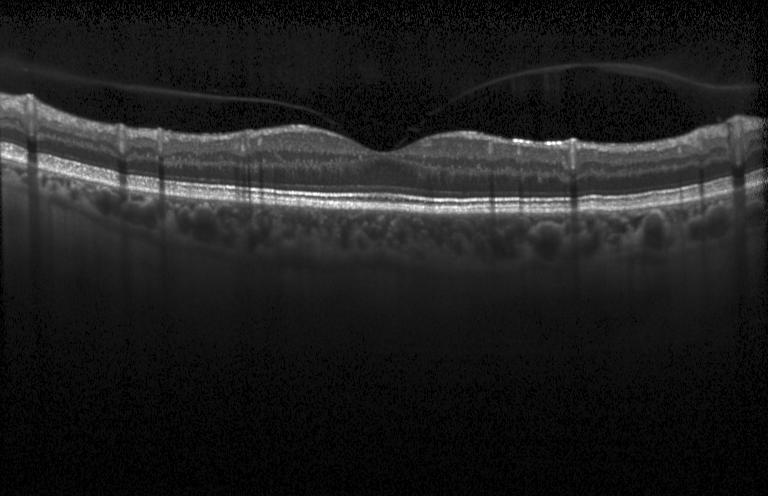
OCT line scan, spectral-domain optical coherence tomography, instrument: Heidelberg Spectralis, fovea-centered.
The scan shows no evidence of CNV, DME, or drusen.